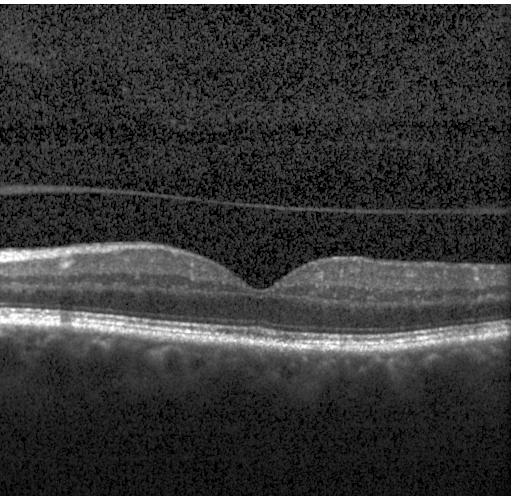 Retinal OCT cross-section. Centered on the fovea — The scan shows no choroidal neovascularization, diabetic macular edema, or drusen.